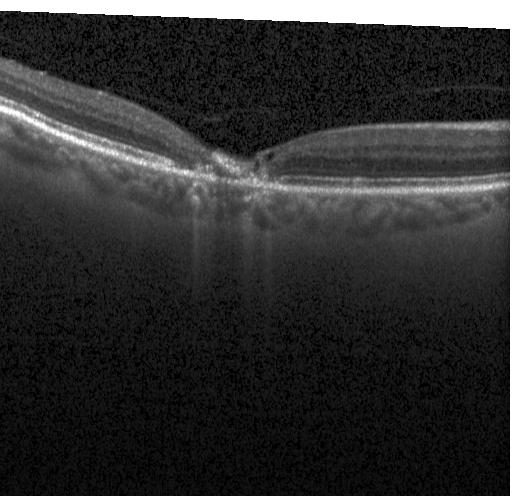
Horizontal scan through the fovea · optical coherence tomography B-scan. Diagnosis: choroidal neovascularization (CNV).